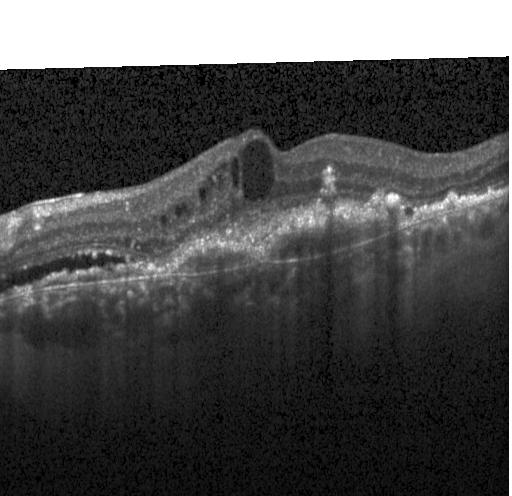
SD-OCT · retinal OCT cross-section · through the macula
Finding: choroidal neovascularization (CNV).